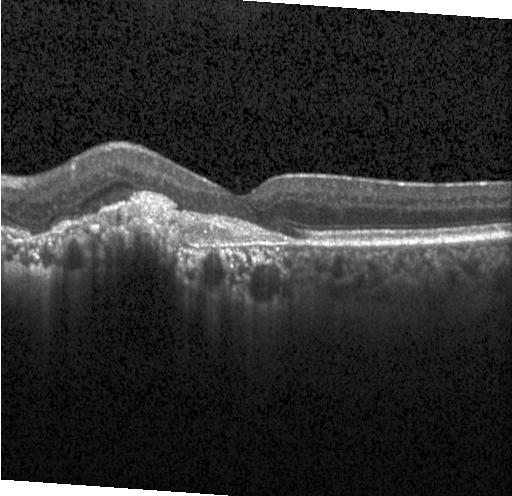 Retinal OCT B-scan. This B-scan demonstrates a choroidal neovascular membrane.